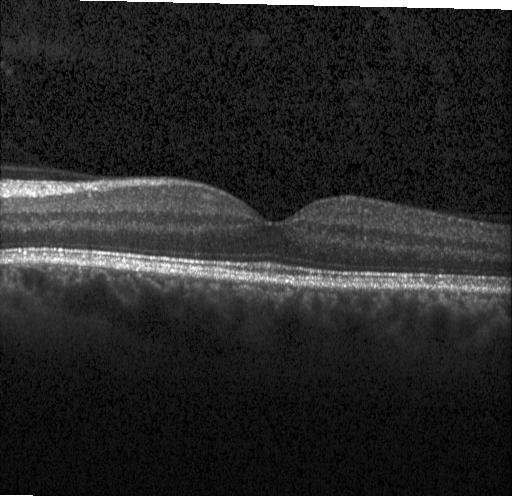 Diagnosis: no evidence of choroidal neovascularization, diabetic macular edema, or drusen.